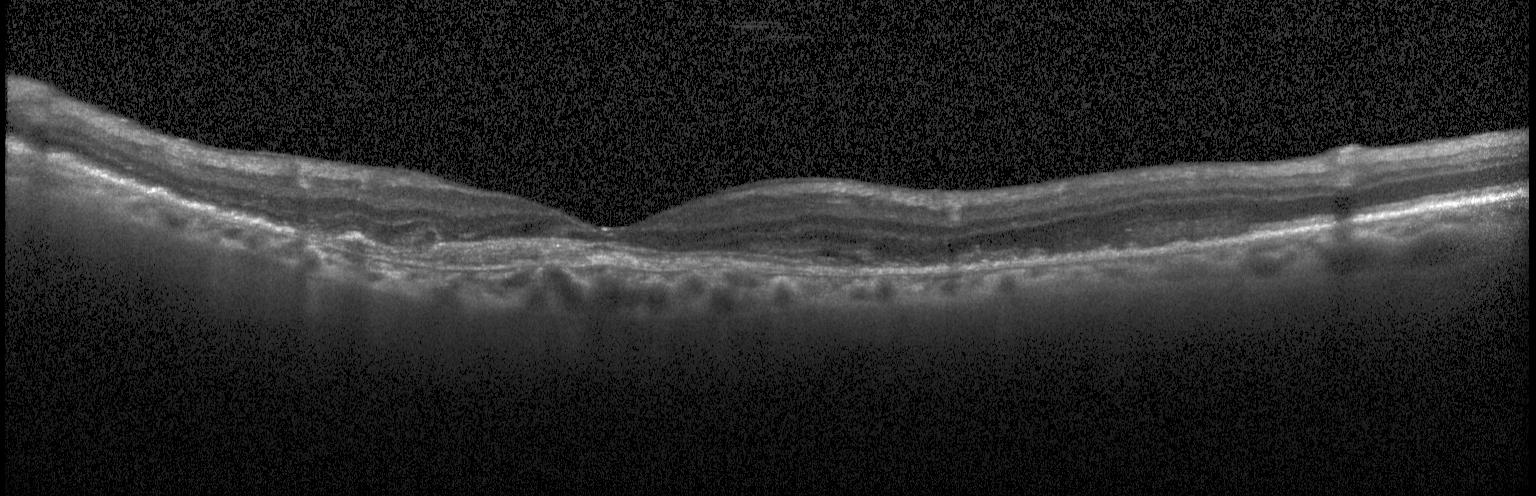
Fovea-centered · retinal OCT B-scan.
Finding: choroidal neovascularization.